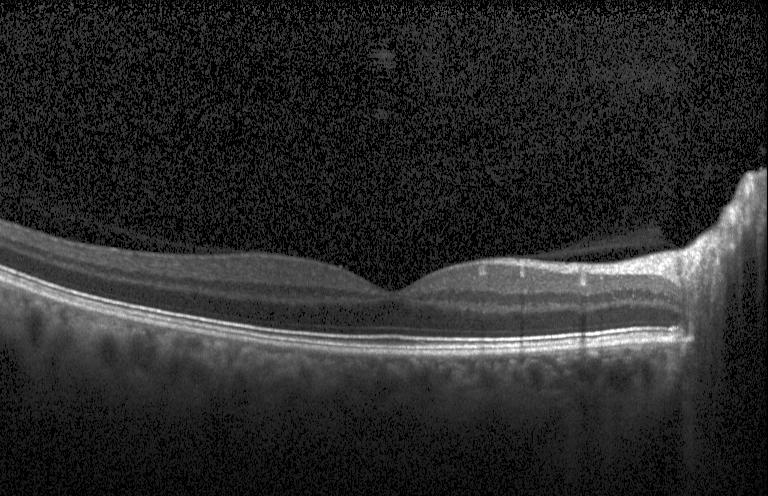 SD-OCT · retinal OCT cross-section. Finding: no CNV, DME, or drusen.